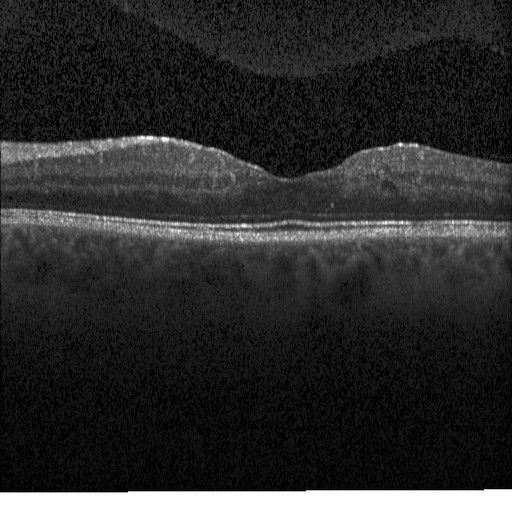 Retinal OCT cross-section showing diabetic macular edema.